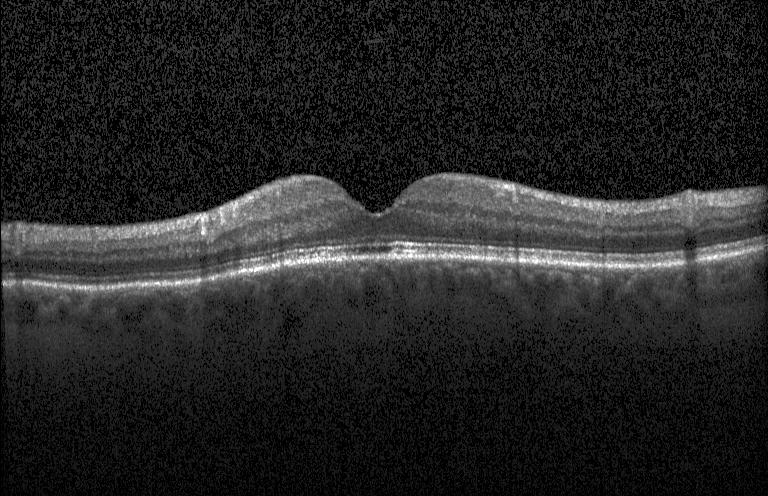 Impression: no evidence of choroidal neovascularization, diabetic macular edema, or drusen.